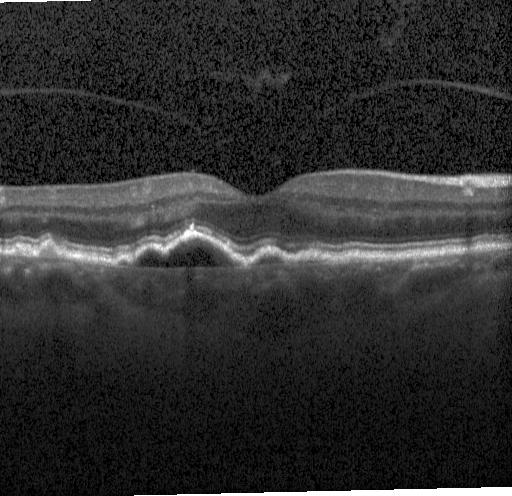 Diagnosis: a choroidal neovascular membrane.